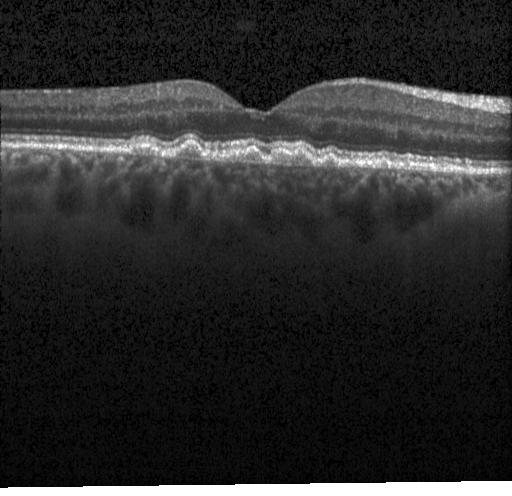
Through the macula; OCT line scan; spectral-domain optical coherence tomography
Finding: sub-RPE drusenoid deposits.